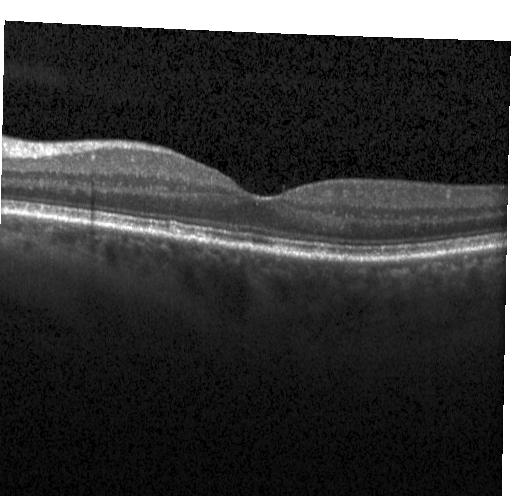 OCT B-scan showing no evidence of choroidal neovascularization, diabetic macular edema, or drusen.